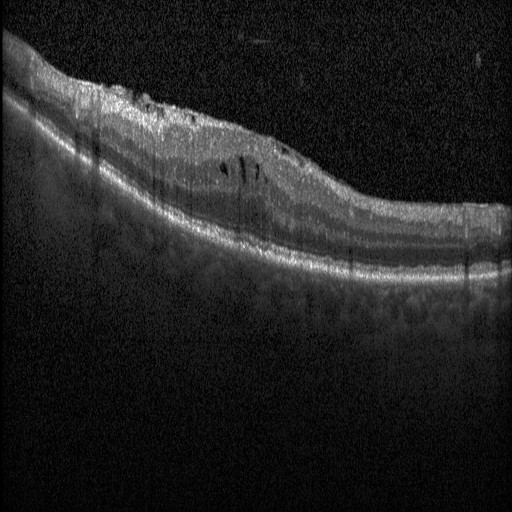

Retinal OCT cross-section. Diabetic macular edema.